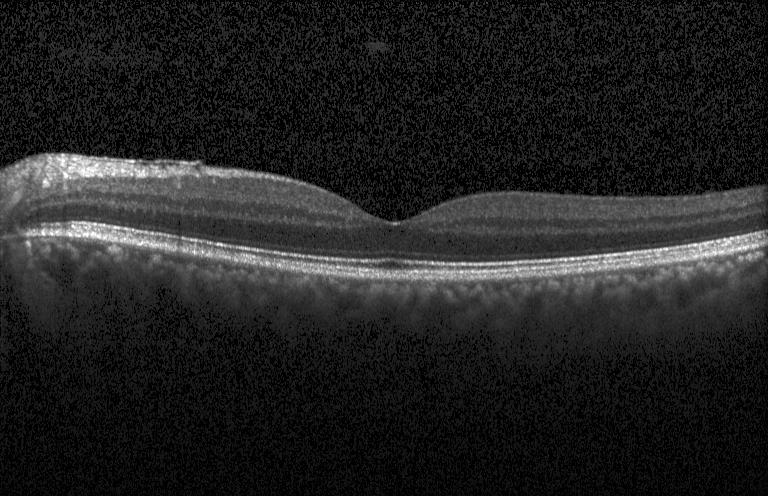 Horizontal scan through the fovea. Optical coherence tomography scan. SD-OCT. Heidelberg Spectralis — Finding: no CNV, no DME, and no drusen.